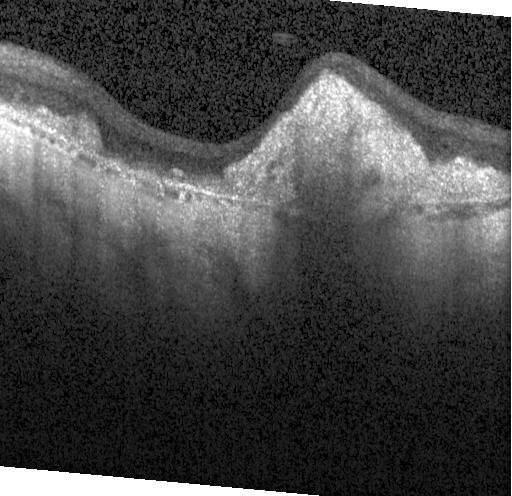

Retinal OCT cross-section. Horizontal scan through the fovea.
Impression: a choroidal neovascular membrane.